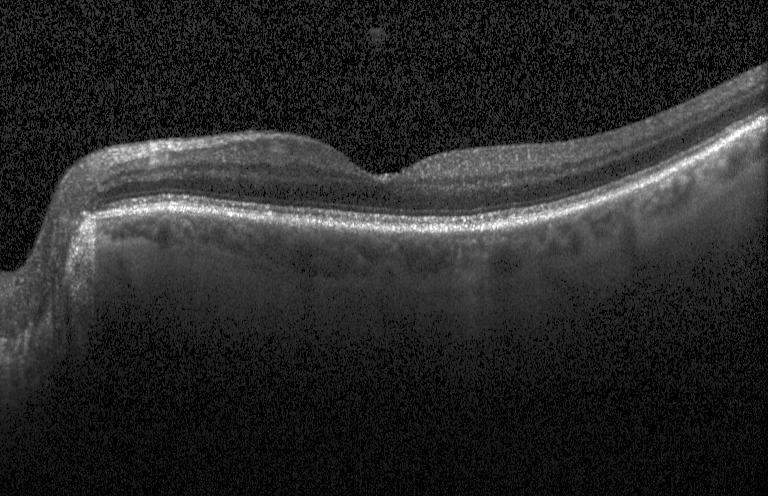 OCT finding: no CNV, no DME, and no drusen.